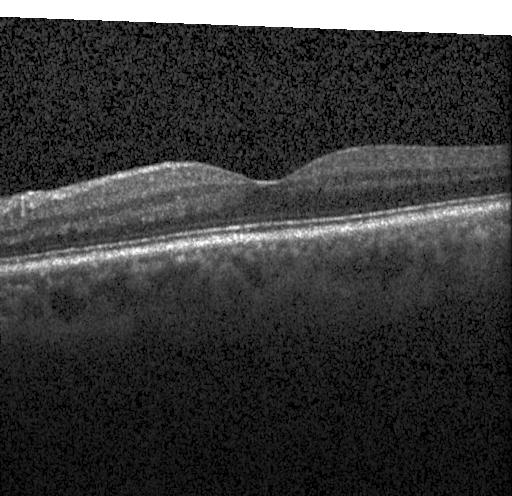
Optical coherence tomography B-scan. Macular scan — The scan shows no choroidal neovascularization, diabetic macular edema, or drusen.